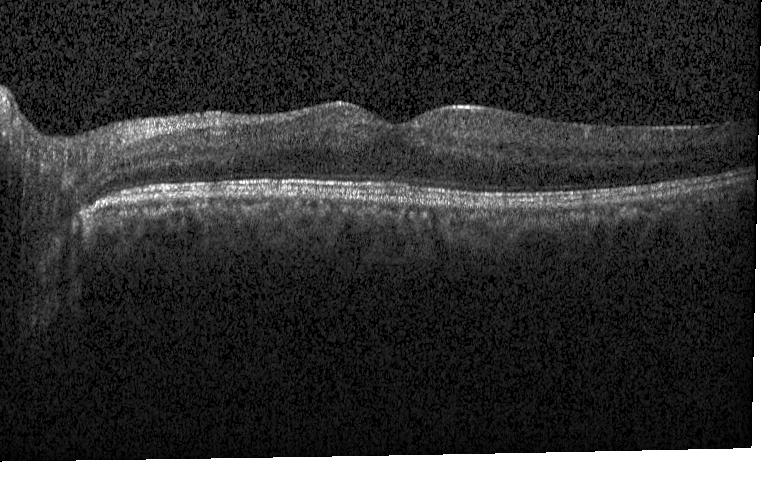
Spectral-domain optical coherence tomography; retinal OCT cross-section; macular scan; instrument: Heidelberg Spectralis.
No choroidal neovascularization, no diabetic macular edema, and no drusen.